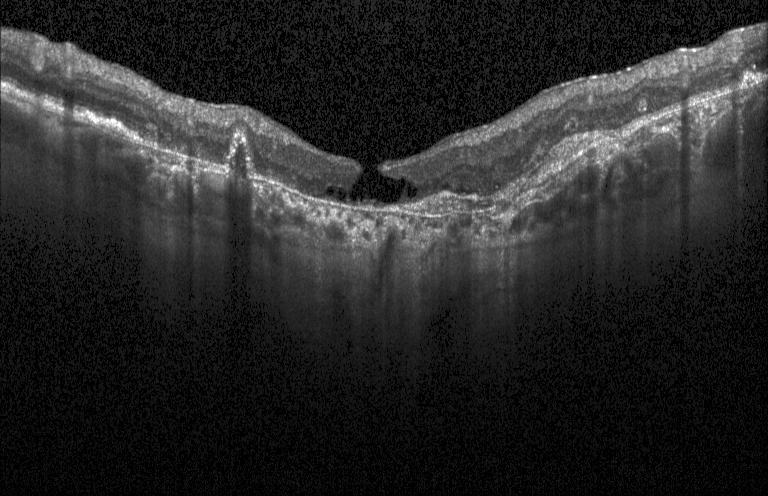
Horizontal scan through the fovea, OCT line scan. This B-scan demonstrates choroidal neovascularization (CNV).